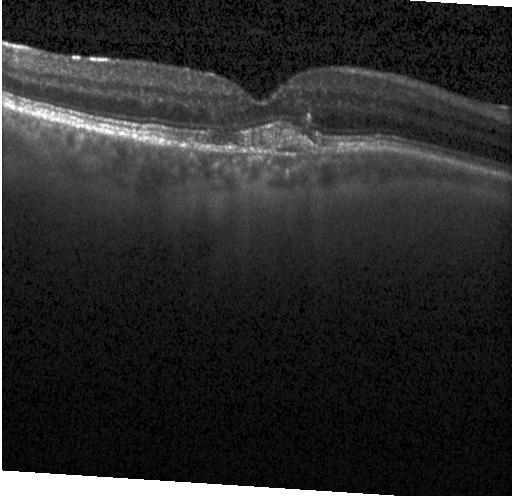 Impression: choroidal neovascularization.